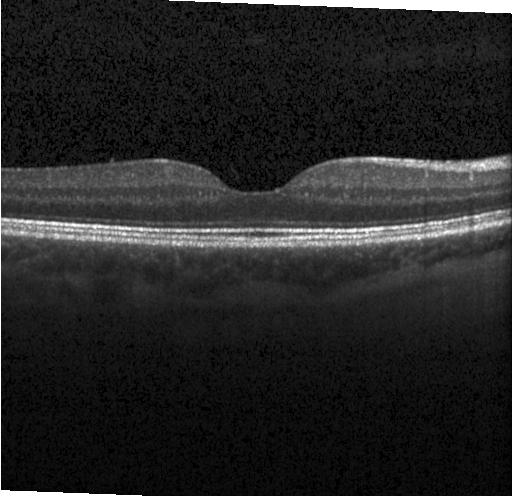

Retinal OCT cross-section, spectral-domain OCT, Heidelberg Spectralis OCT system
The scan shows neither choroidal neovascularization, diabetic macular edema, nor drusen.